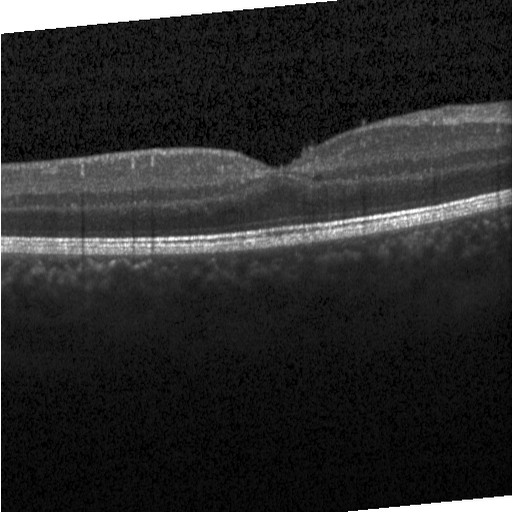 Retinal OCT cross-section. Finding: diabetic macular edema (DME).